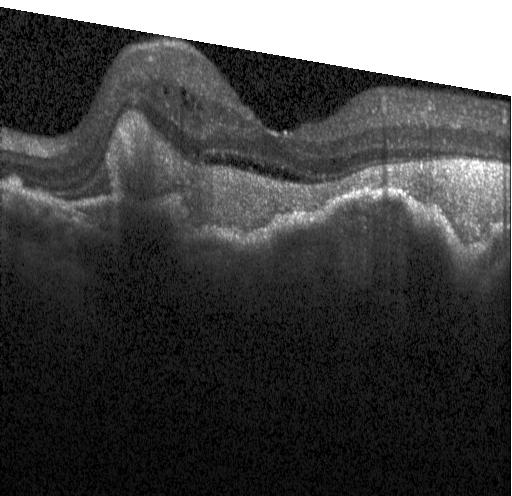 Retinal OCT B-scan — Diagnosis: a choroidal neovascular membrane.